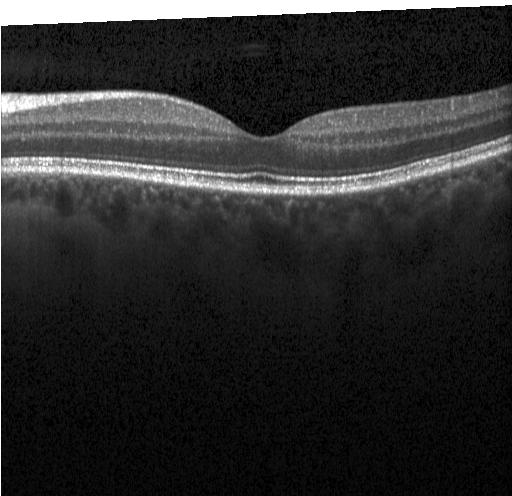 Retinal OCT cross-section showing neither choroidal neovascularization, diabetic macular edema, nor drusen.